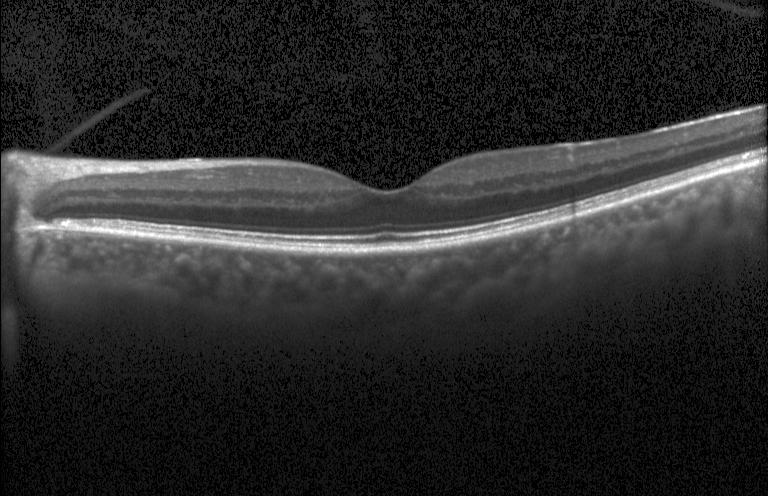
Retinal OCT cross-section. Centered on the fovea. SD-OCT — No CNV, no DME, and no drusen.